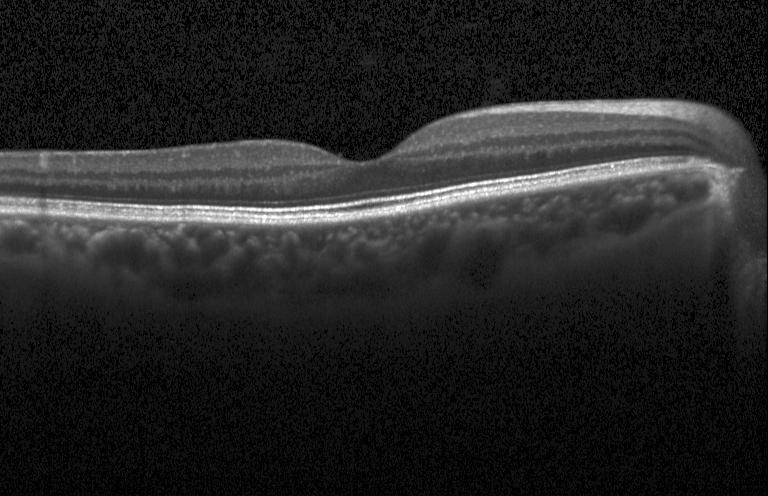

OCT B-scan. Acquired on a Heidelberg Spectralis
Neither choroidal neovascularization, diabetic macular edema, nor drusen.